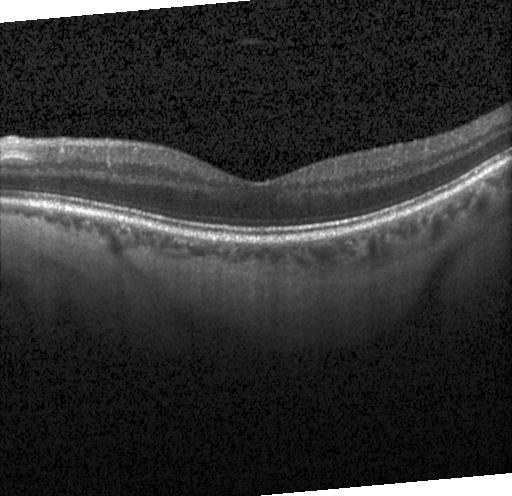 Heidelberg Spectralis · retinal OCT B-scan · through the macula
The scan shows no choroidal neovascularization, no diabetic macular edema, and no drusen.